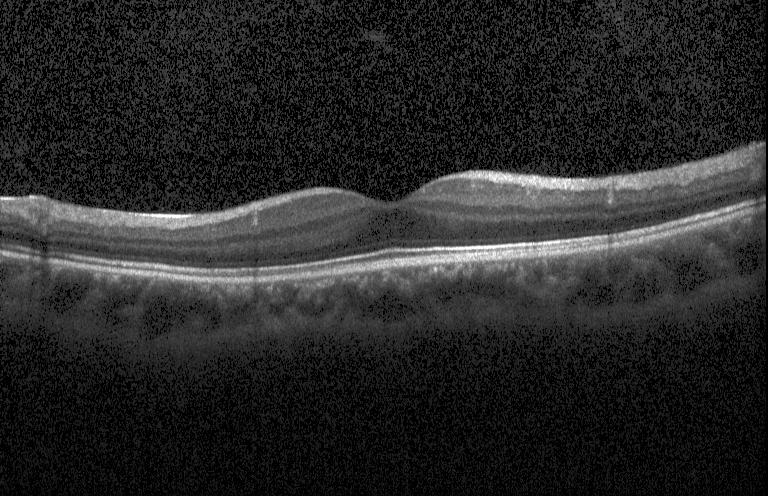 Macular scan; spectral-domain OCT; Heidelberg Spectralis; retinal OCT B-scan.
Impression: neither choroidal neovascularization, diabetic macular edema, nor drusen.